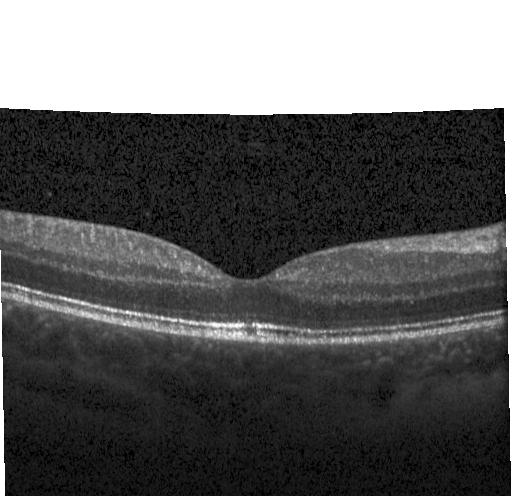

Optical coherence tomography B-scan; macular scan; Heidelberg Spectralis OCT system
Neither CNV, DME, nor drusen.